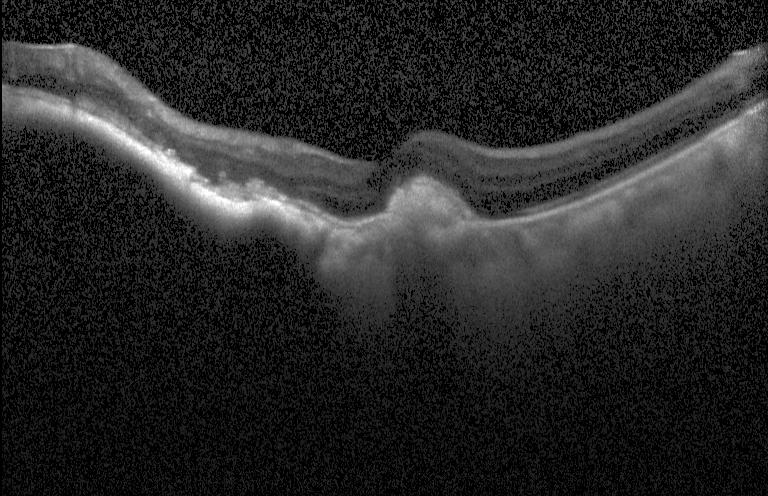 Impression: choroidal neovascularization.